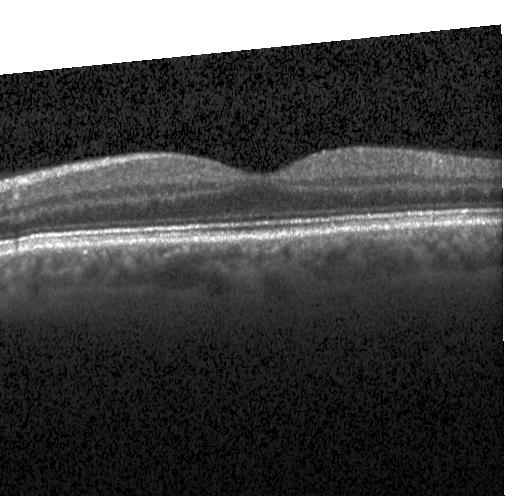

Through the macula. Optical coherence tomography B-scan. Finding: no choroidal neovascularization, no diabetic macular edema, and no drusen.